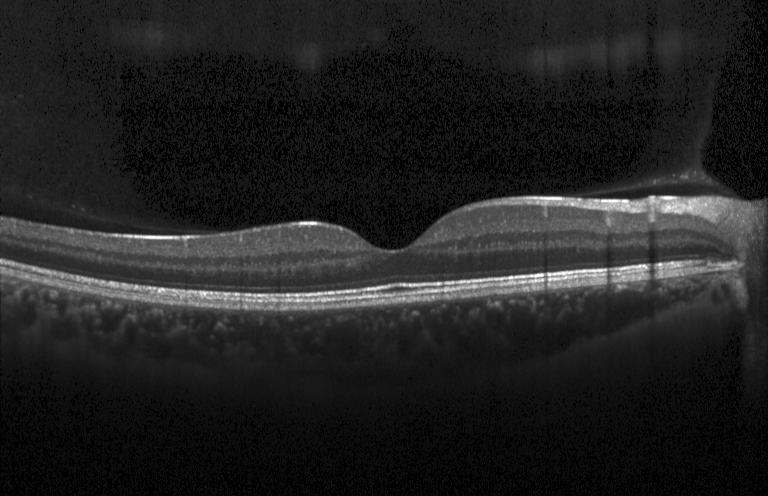
Optical coherence tomography B-scan.
Diagnosis: no CNV, DME, or drusen.